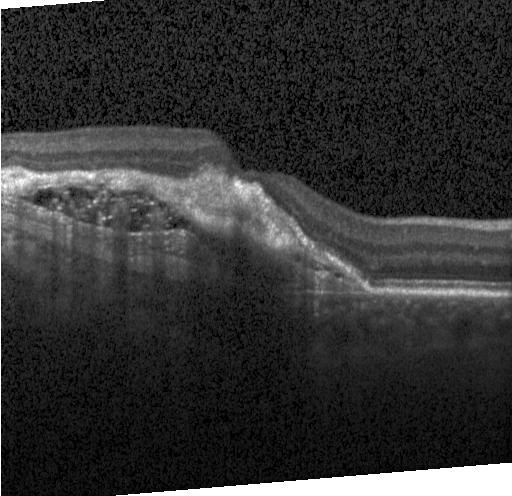

Optical coherence tomography scan — This B-scan demonstrates a choroidal neovascular membrane.